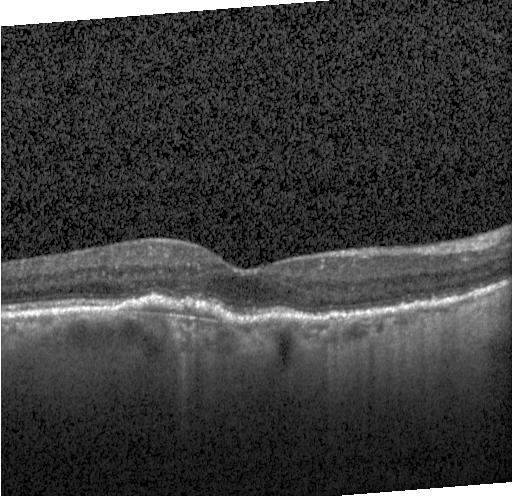 Diagnosis: choroidal neovascularization (CNV).